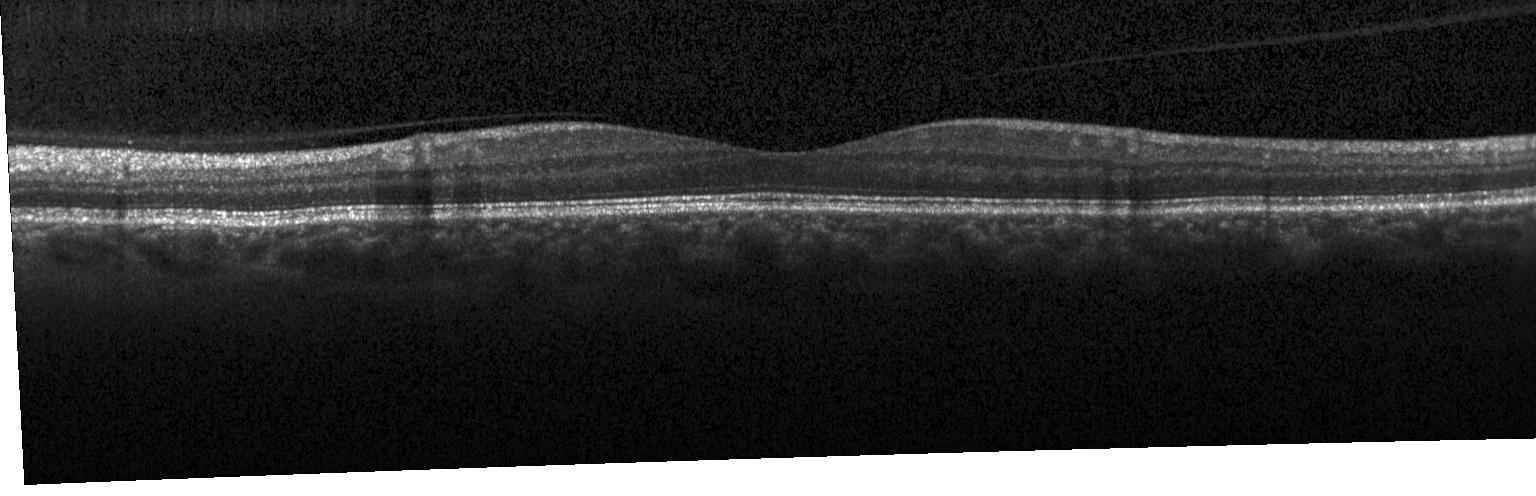 OCT finding: no choroidal neovascularization, diabetic macular edema, or drusen.